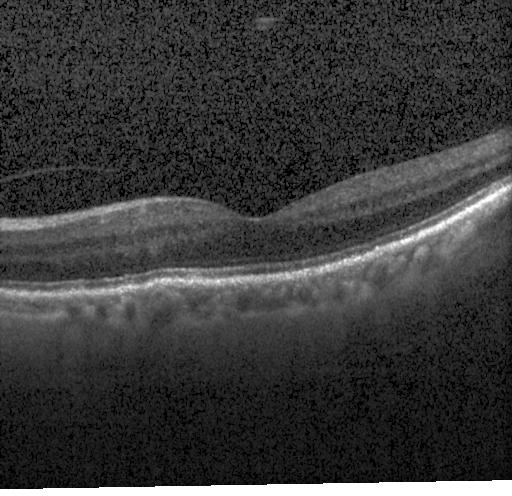 Impression: no choroidal neovascularization, diabetic macular edema, or drusen.